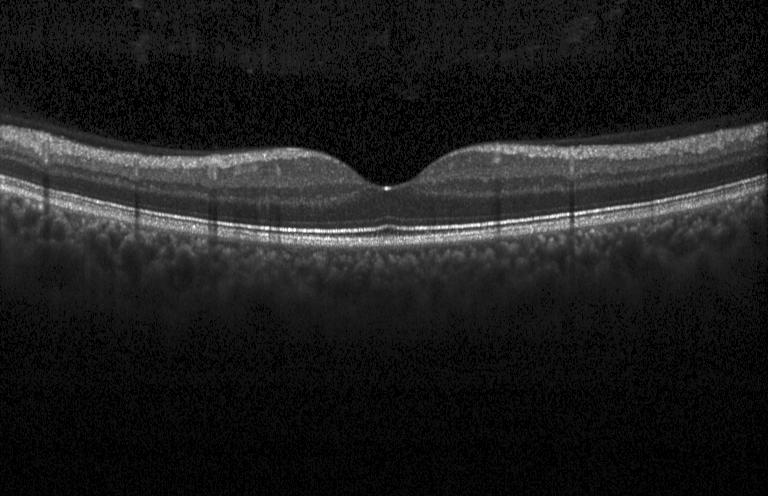

OCT line scan, through the macula.
Diagnosis: no CNV, no DME, and no drusen.